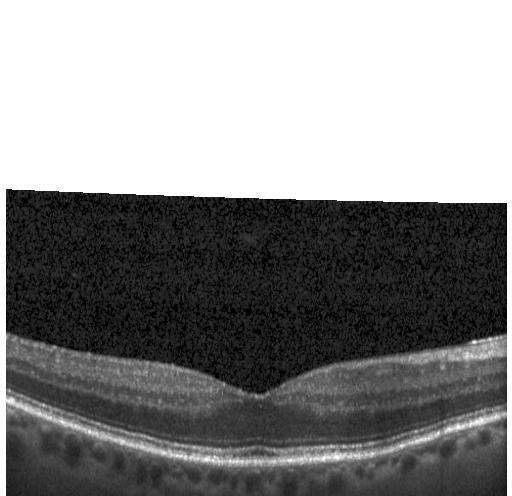 Diagnosis: no CNV, no DME, and no drusen.